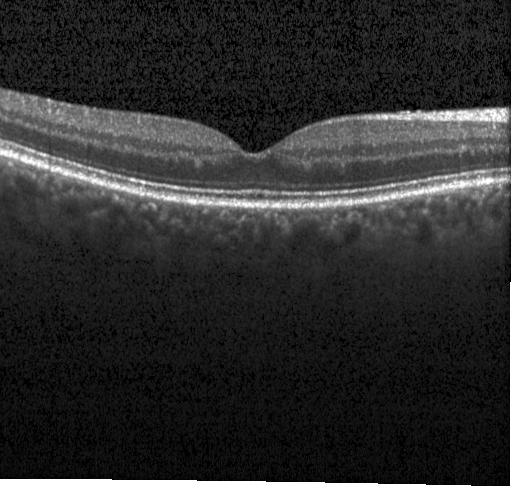 Optical coherence tomography B-scan; spectral-domain optical coherence tomography; Heidelberg Spectralis
Macular OCT: no evidence of choroidal neovascularization, diabetic macular edema, or drusen.